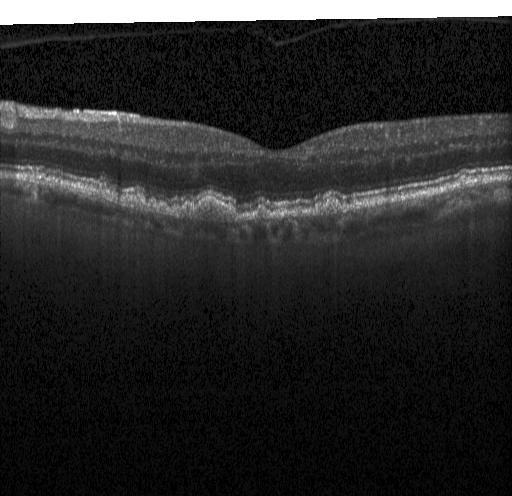
Optical coherence tomography scan, horizontal scan through the fovea. Impression: sub-RPE drusenoid deposits.